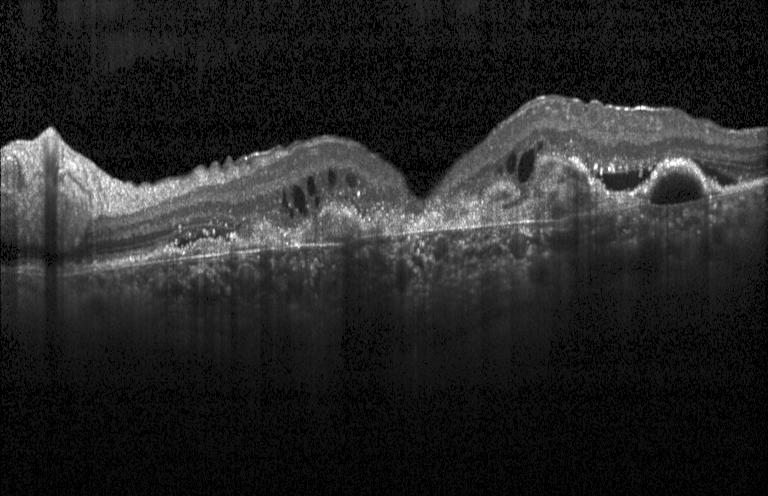

Retinal OCT B-scan, spectral-domain OCT. Finding: a choroidal neovascular membrane.